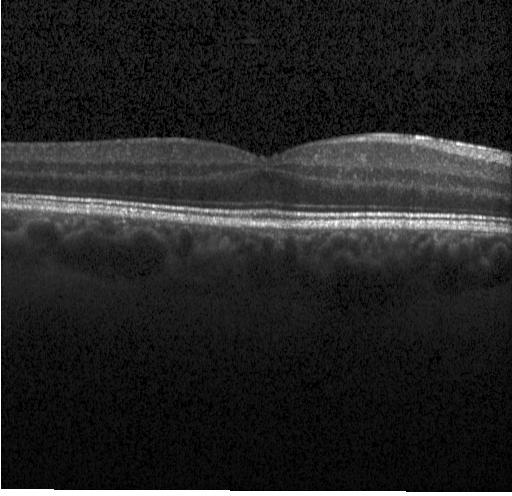
Macular OCT: neither CNV, DME, nor drusen.